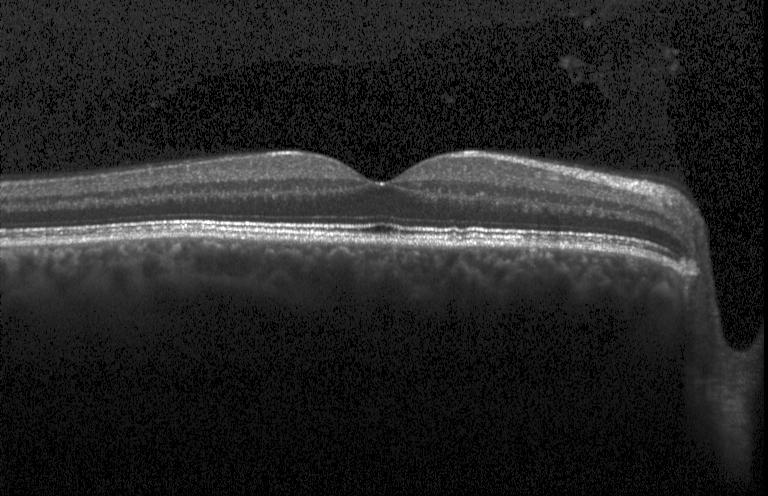 OCT B-scan. This B-scan demonstrates no evidence of choroidal neovascularization, diabetic macular edema, or drusen.